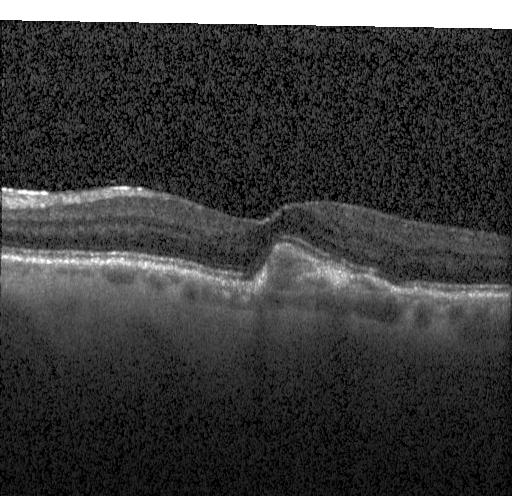

Heidelberg Spectralis · spectral-domain OCT · retinal OCT B-scan.
This B-scan demonstrates a choroidal neovascular membrane.